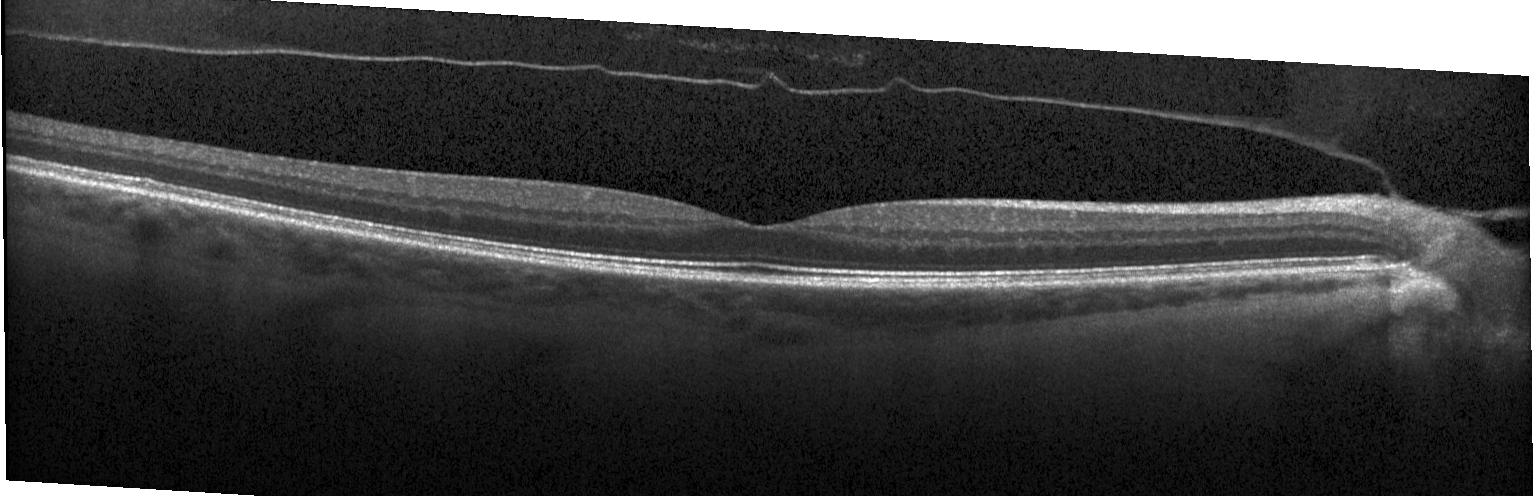 Retinal OCT cross-section.
Assessment: no CNV, no DME, and no drusen.